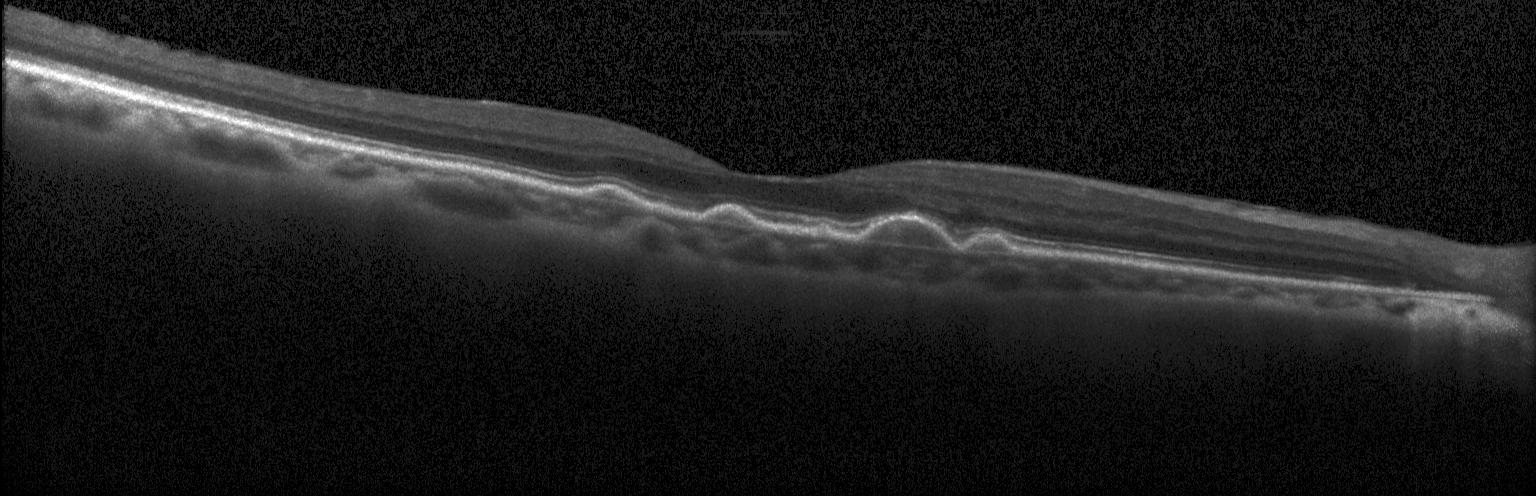

OCT line scan, Heidelberg Spectralis OCT system, through the macula
This B-scan demonstrates drusen.